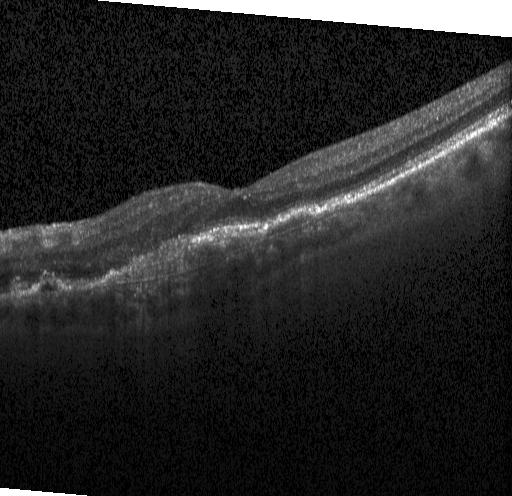

Heidelberg Spectralis OCT system. Optical coherence tomography scan.
Assessment: CNV.